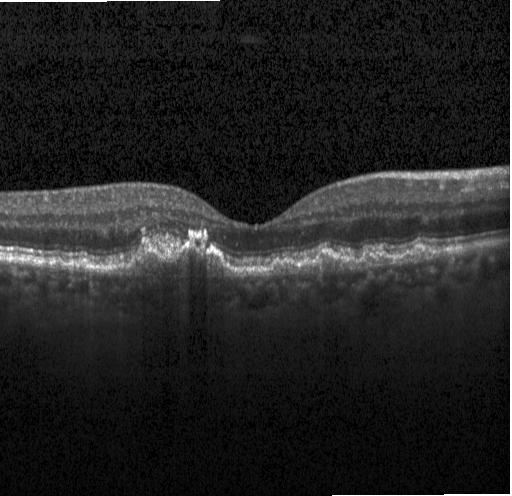

The scan shows CNV.